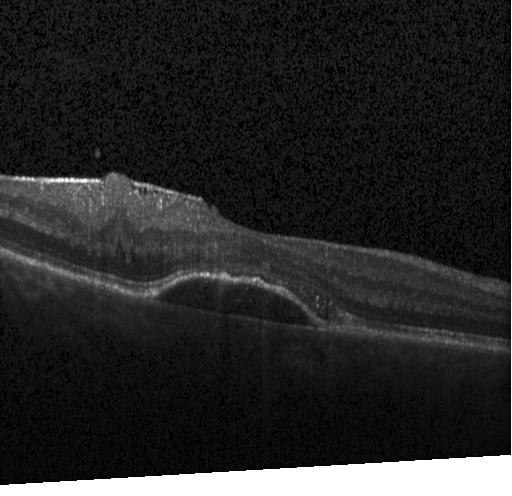

OCT finding: choroidal neovascularization (CNV).